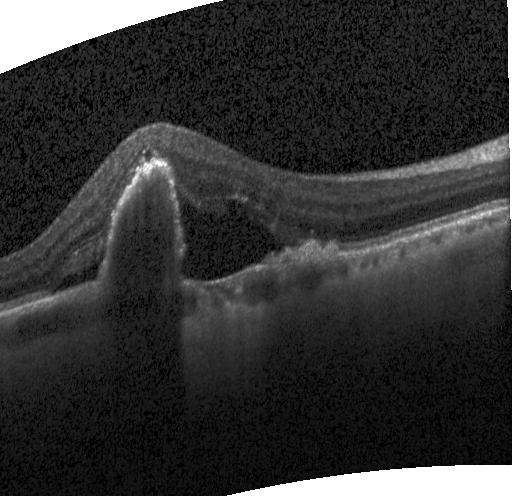
Through the macula · SD-OCT · optical coherence tomography B-scan · acquired on a Heidelberg Spectralis. Diagnosis: choroidal neovascularization.